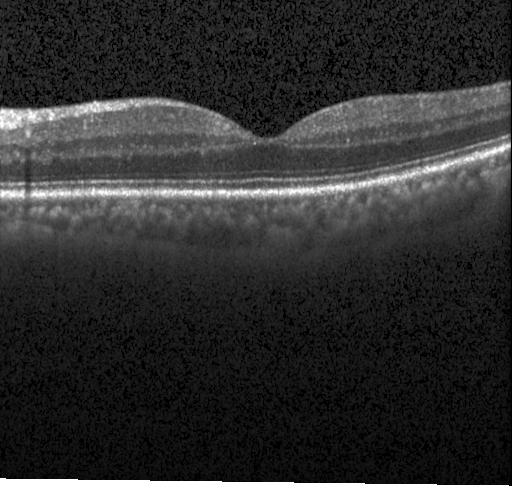 Optical coherence tomography scan · fovea-centered.
Dx: neither CNV, DME, nor drusen.